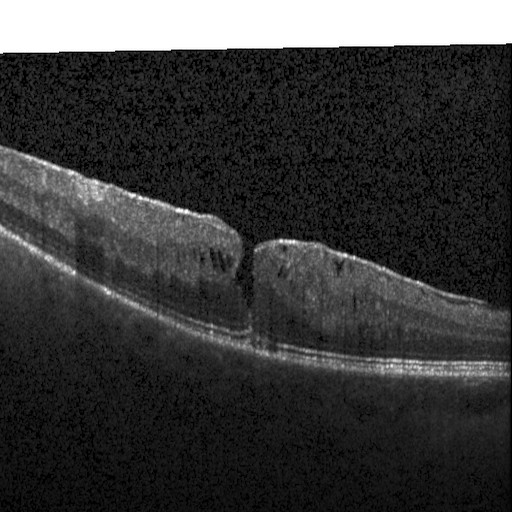 Dx: DME.